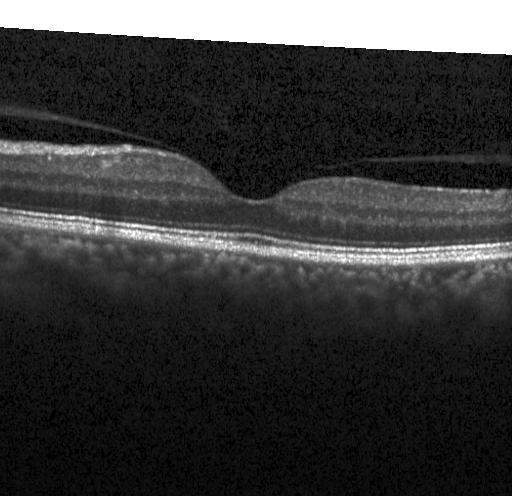 Assessment: no choroidal neovascularization, no diabetic macular edema, and no drusen.